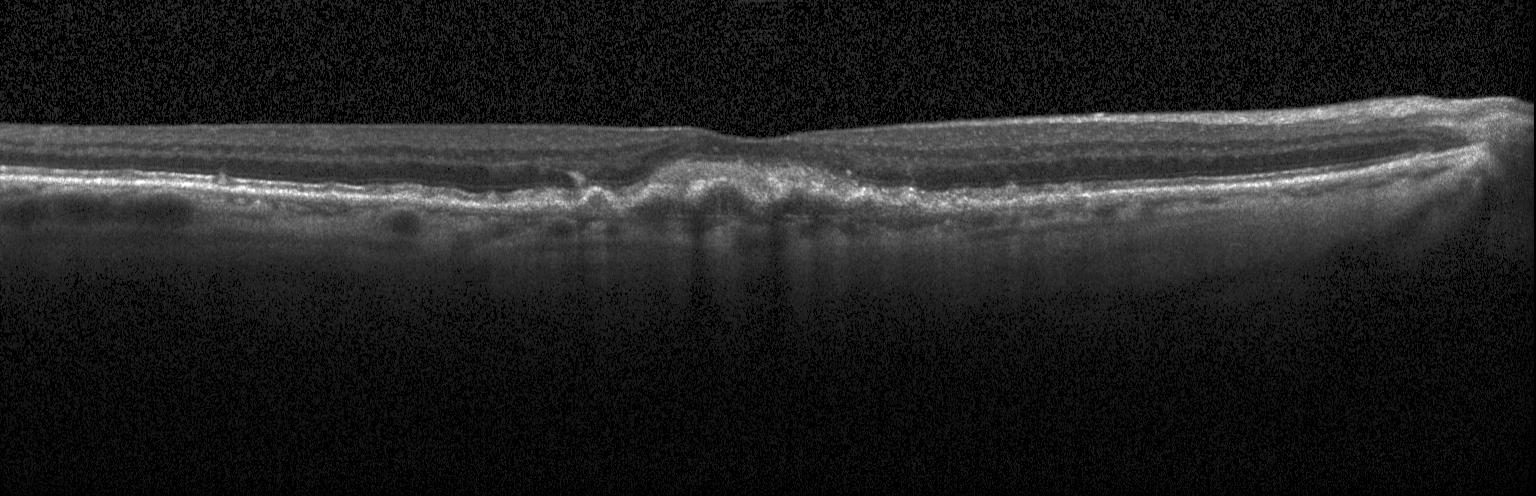
Centered on the fovea; Heidelberg Spectralis; SD-OCT; optical coherence tomography scan — Choroidal neovascularization.